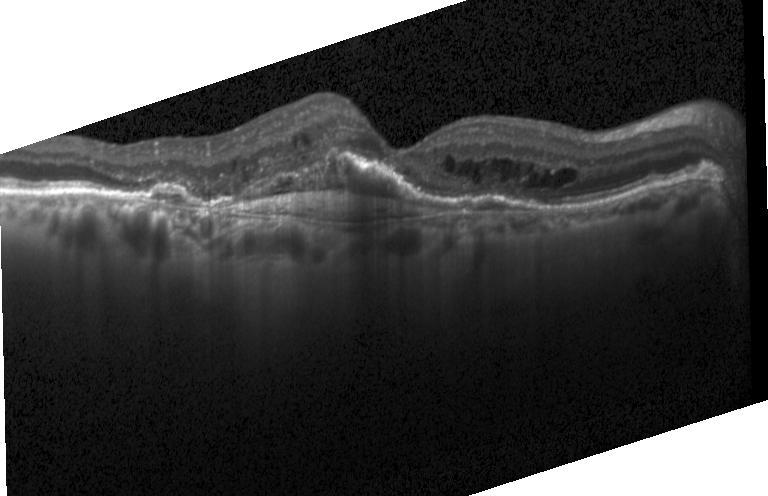

Impression: CNV.